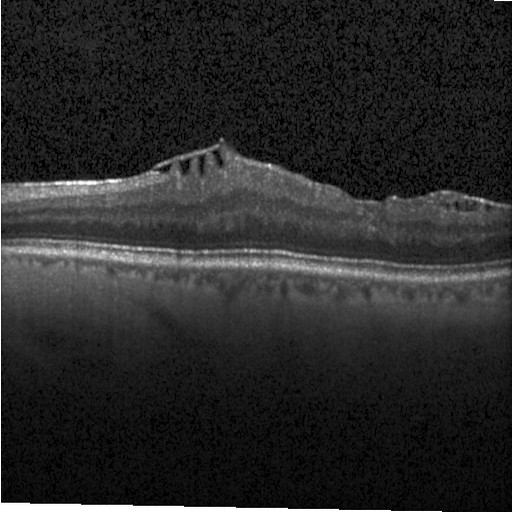
Retinal OCT cross-section; SD-OCT
Impression: diabetic macular edema (DME).